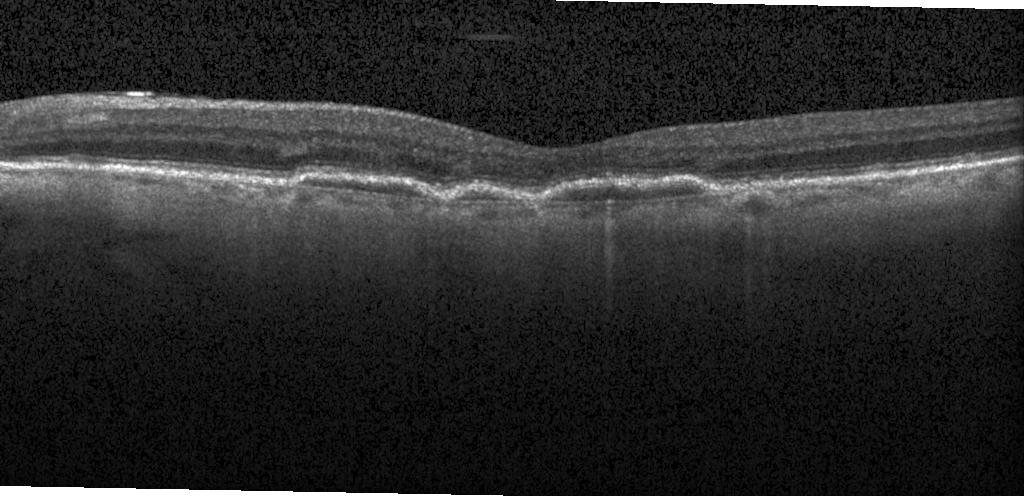 Impression: CNV.